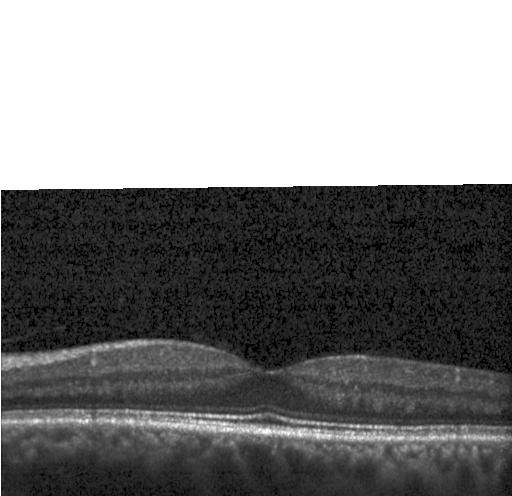
Heidelberg Spectralis · fovea-centered · optical coherence tomography scan — No choroidal neovascularization, no diabetic macular edema, and no drusen.